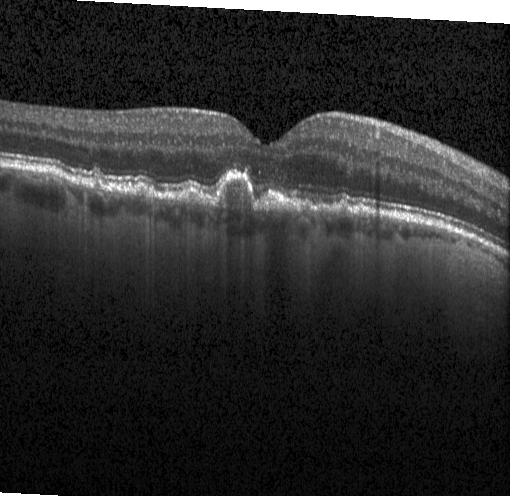 OCT line scan. Impression: drusen.